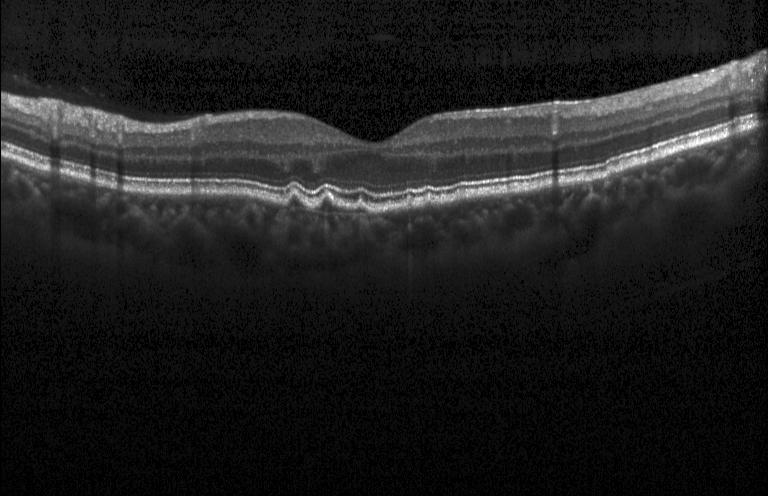

Optical coherence tomography B-scan; macular scan; SD-OCT; Heidelberg Spectralis OCT system
Dx: multiple drusen.